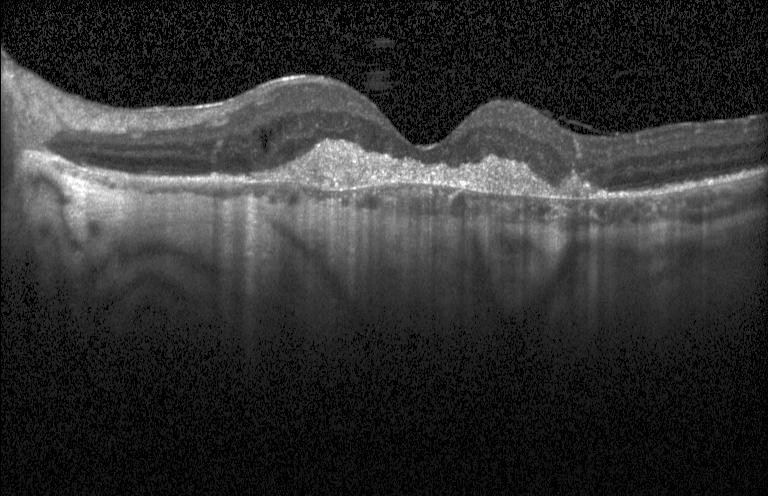
Spectral-domain OCT B-scan: CNV.